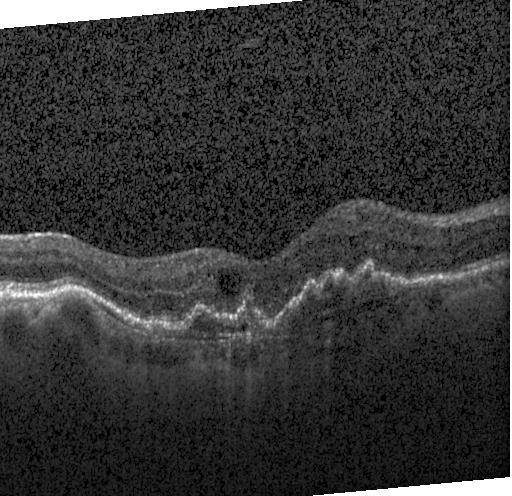

Retinal OCT cross-section showing choroidal neovascularization (CNV).